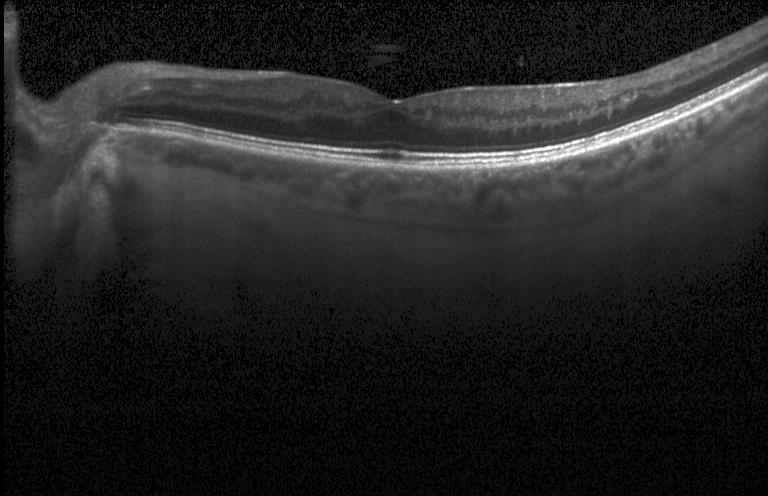
Retinal OCT B-scan.
Neither choroidal neovascularization, diabetic macular edema, nor drusen.